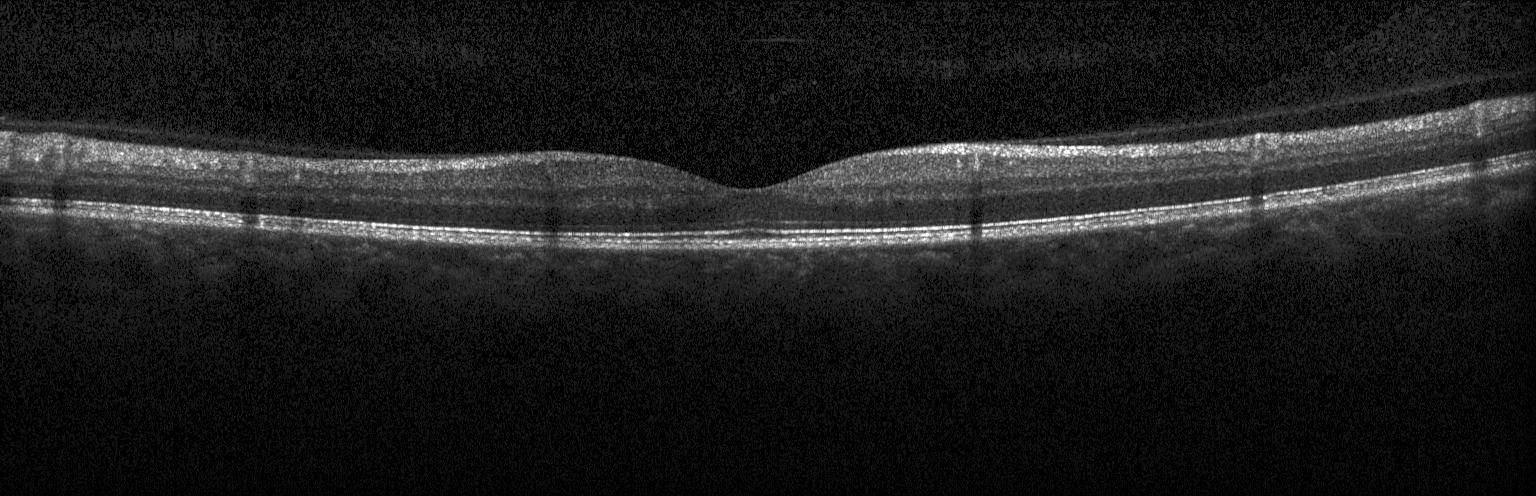
Spectral-domain OCT B-scan: neither choroidal neovascularization, diabetic macular edema, nor drusen.